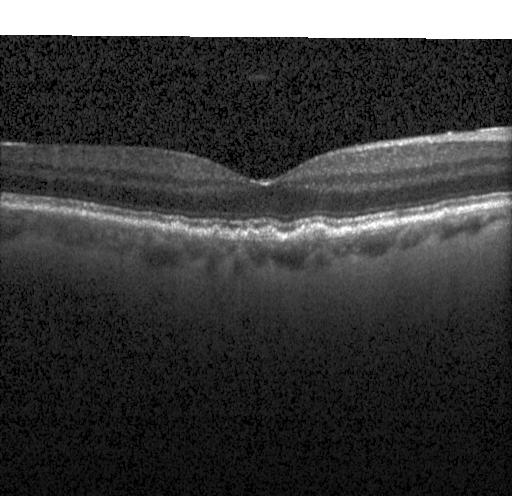
Optical coherence tomography B-scan · macular scan.
Multiple drusen.